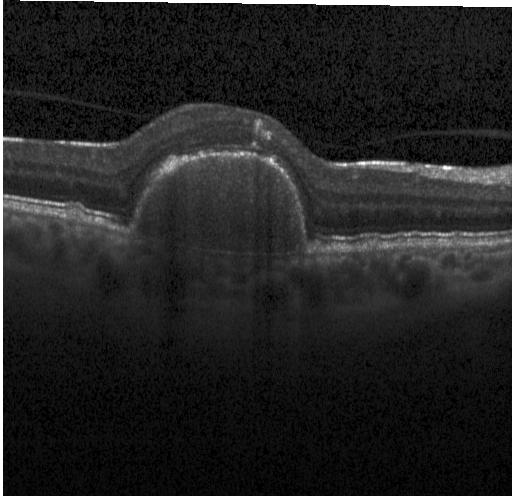

Spectral-domain OCT B-scan: choroidal neovascularization (CNV).